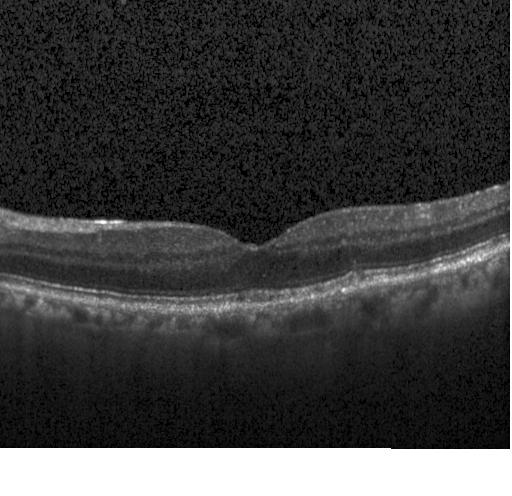
OCT finding: drusen.